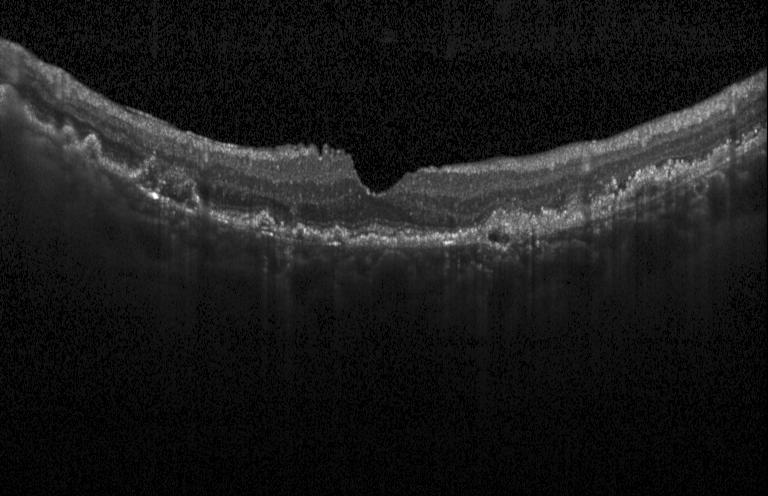

Diagnosis: CNV.